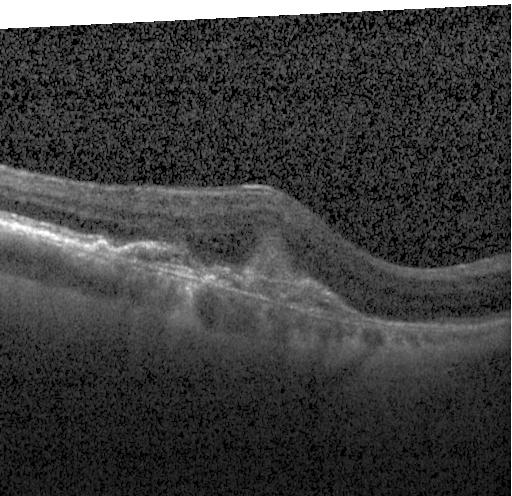

Diagnosis: a choroidal neovascular membrane.